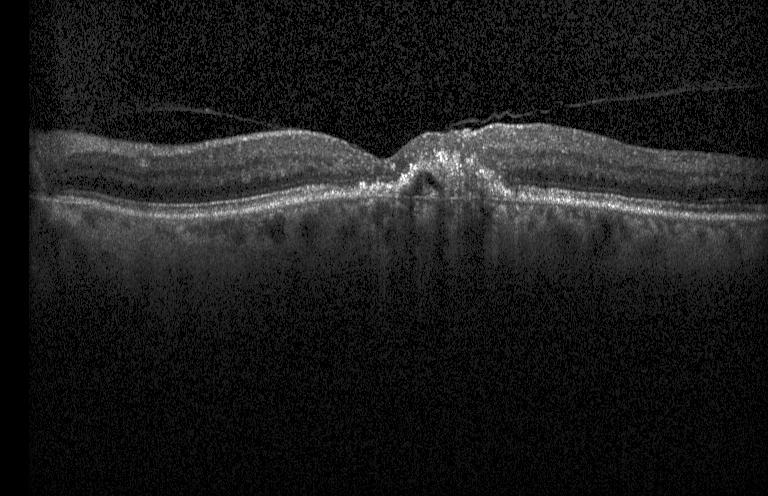

OCT B-scan.
Assessment: a choroidal neovascular membrane.